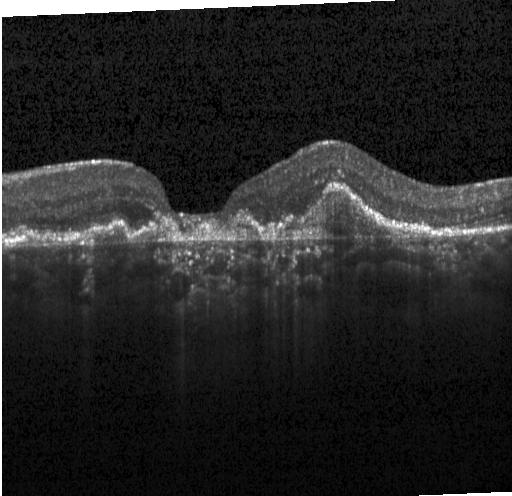 Optical coherence tomography B-scan. This B-scan demonstrates a choroidal neovascular membrane.